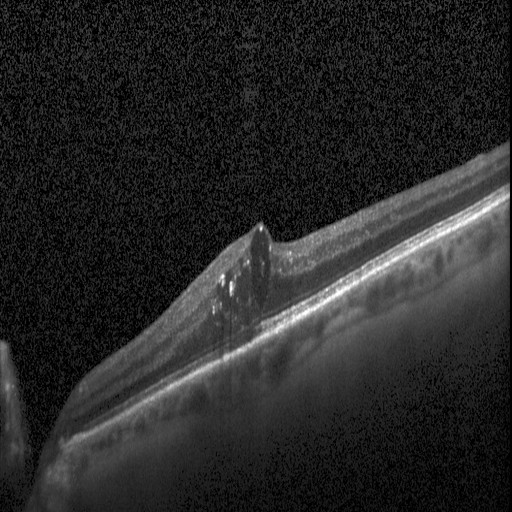 Fovea-centered. Optical coherence tomography scan. Acquired on a Heidelberg Spectralis. Dx: diabetic macular edema.